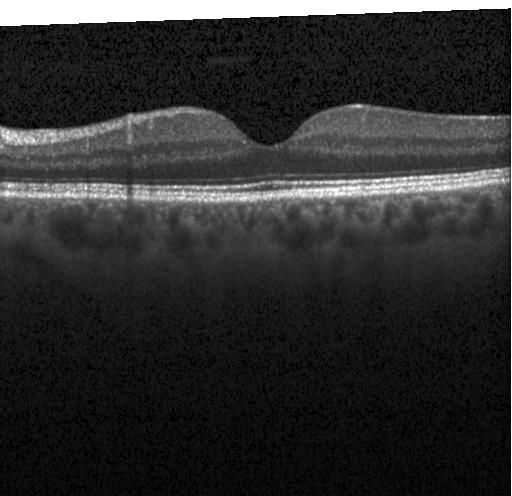

Fovea-centered · retinal OCT B-scan — Finding: no evidence of choroidal neovascularization, diabetic macular edema, or drusen.